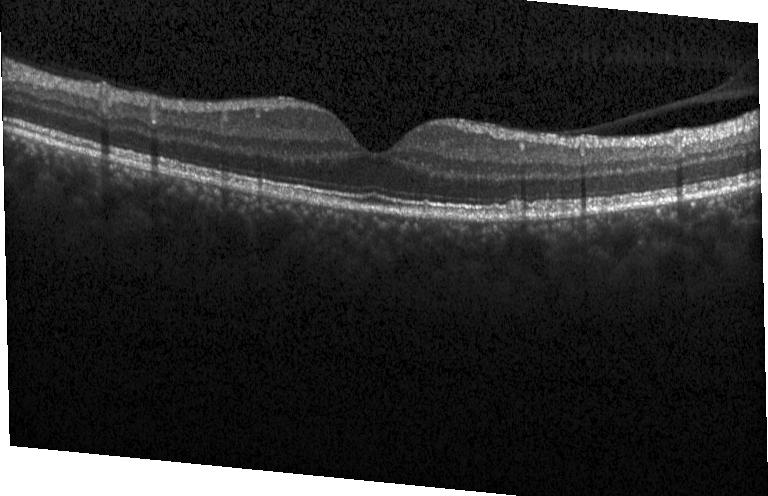

Heidelberg Spectralis OCT system. Centered on the fovea. Optical coherence tomography scan — Diagnosis: no CNV, DME, or drusen.